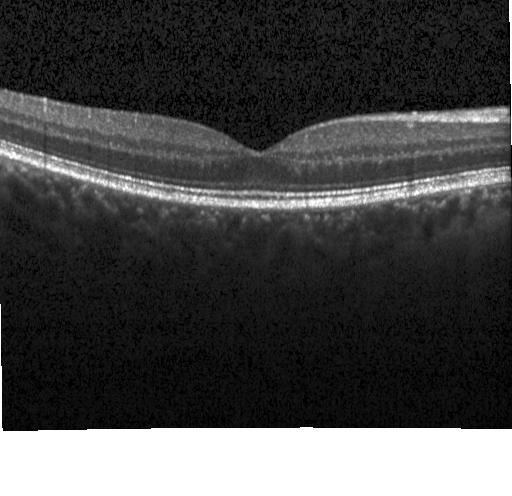
Spectral-domain OCT B-scan: no evidence of CNV, DME, or drusen.